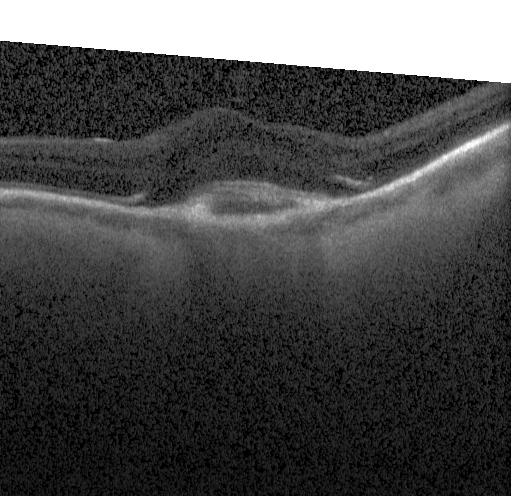
Optical coherence tomography B-scan, spectral-domain optical coherence tomography
This B-scan demonstrates a choroidal neovascular membrane.